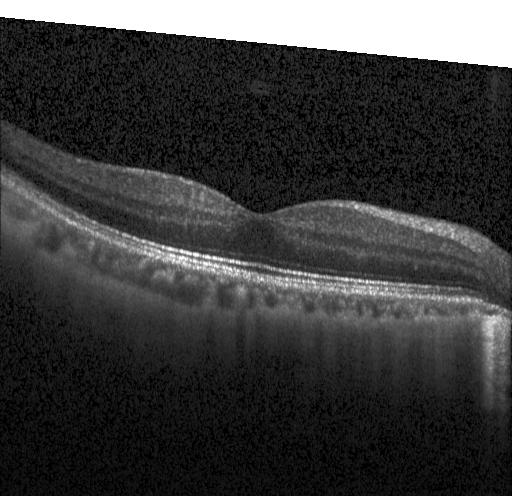
Diagnosis: neither choroidal neovascularization, diabetic macular edema, nor drusen.